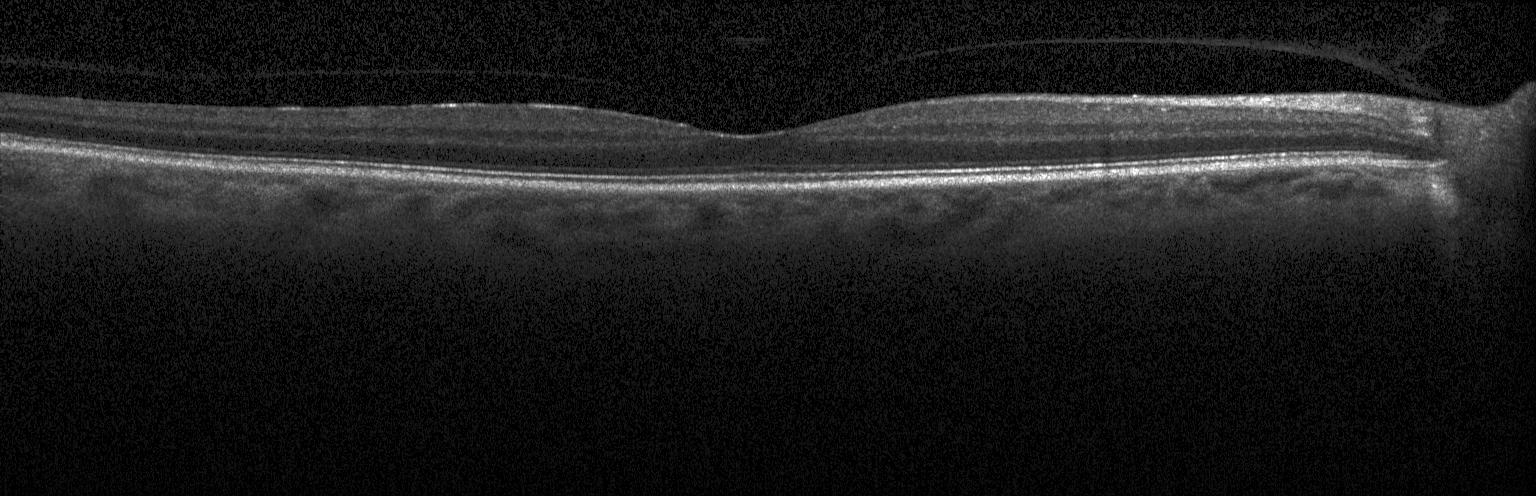 Impression: no choroidal neovascularization, diabetic macular edema, or drusen.